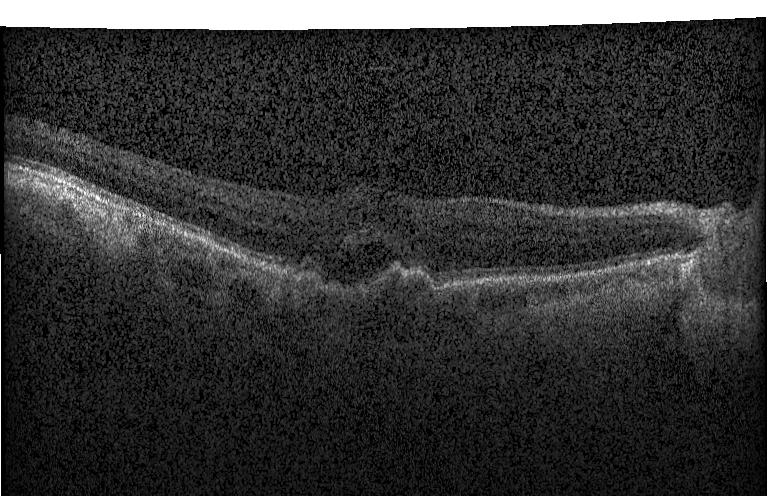

Horizontal scan through the fovea; SD-OCT; OCT B-scan.
Assessment: CNV.